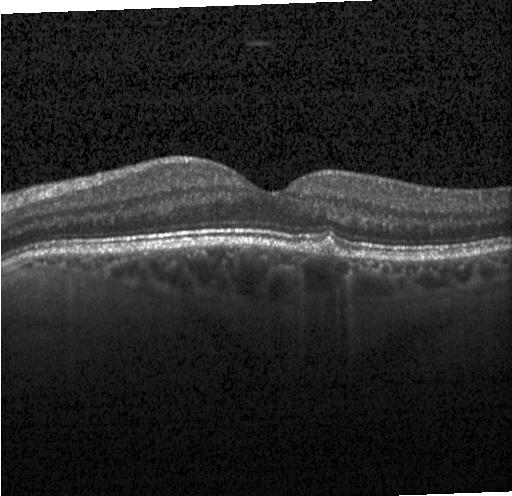
Fovea-centered · optical coherence tomography scan. Impression: multiple drusen.